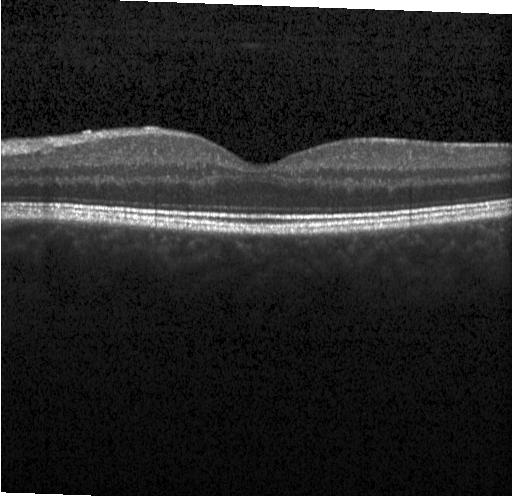 Macular OCT: neither choroidal neovascularization, diabetic macular edema, nor drusen.